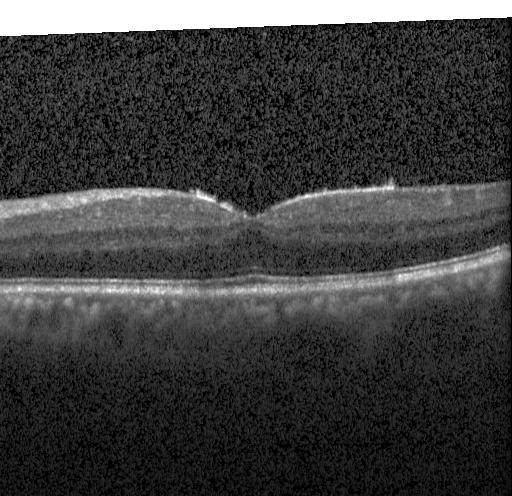 Retinal OCT cross-section · through the macula · SD-OCT
OCT finding: neither choroidal neovascularization, diabetic macular edema, nor drusen.